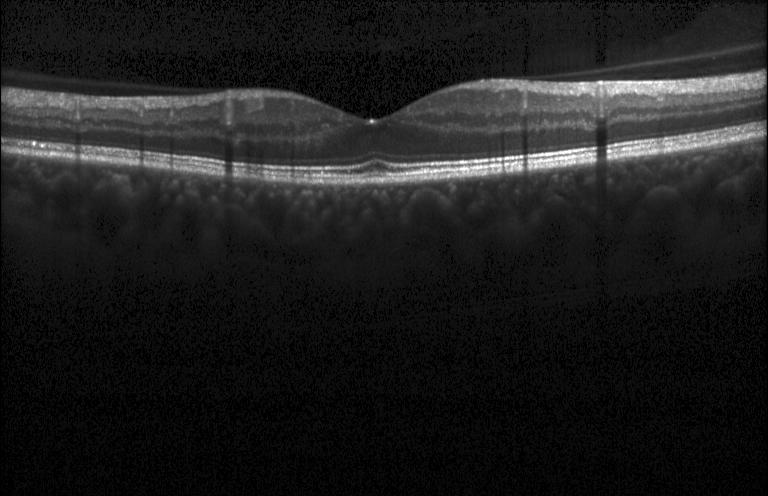
Finding: no evidence of choroidal neovascularization, diabetic macular edema, or drusen.